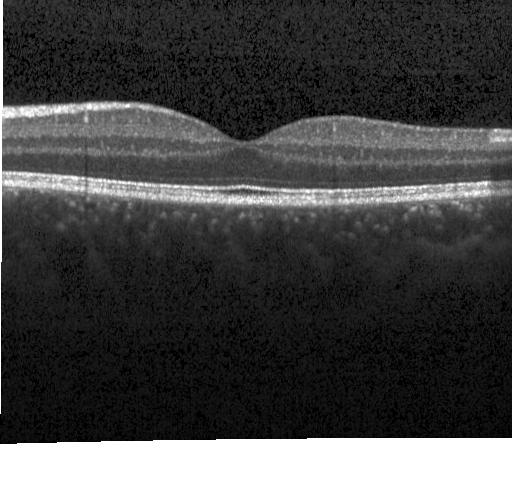 Impression: no evidence of choroidal neovascularization, diabetic macular edema, or drusen.